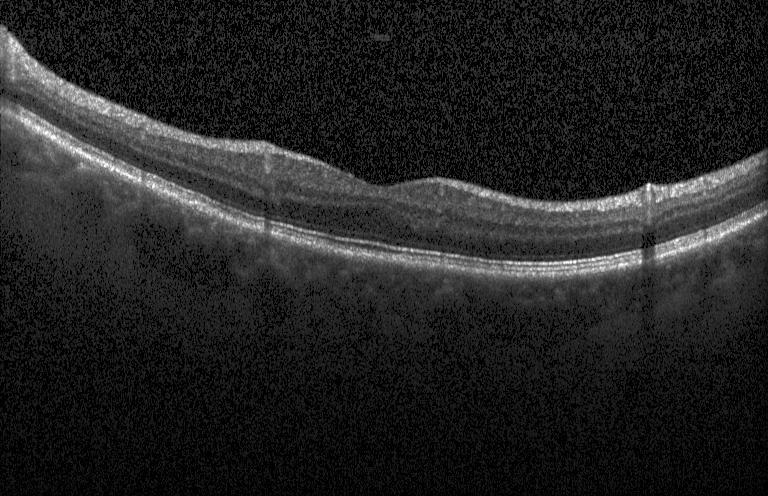 Diagnosis: no CNV, no DME, and no drusen.